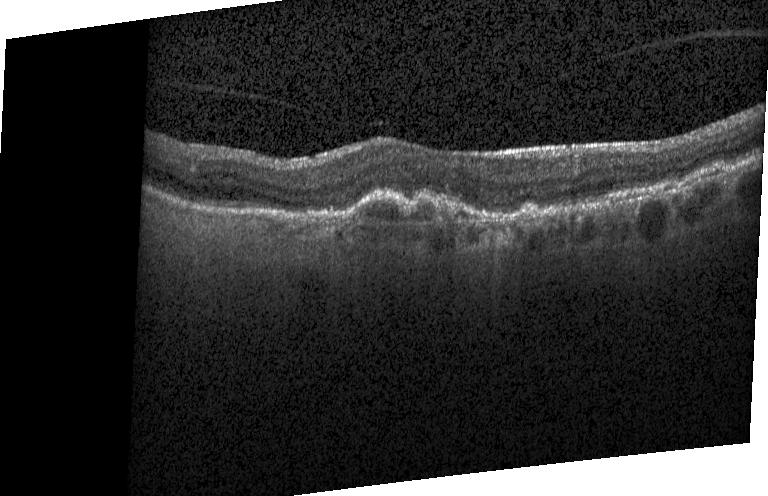
OCT finding: choroidal neovascularization.